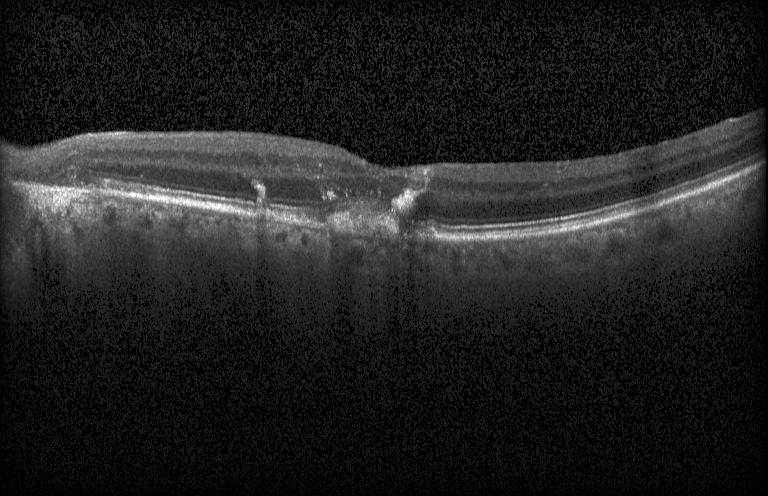 Fovea-centered. Optical coherence tomography B-scan
Impression: choroidal neovascularization (CNV).